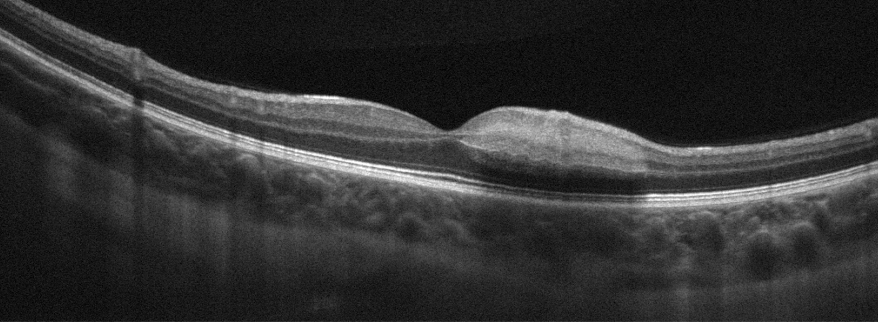 Assessment: retinal artery occlusion.